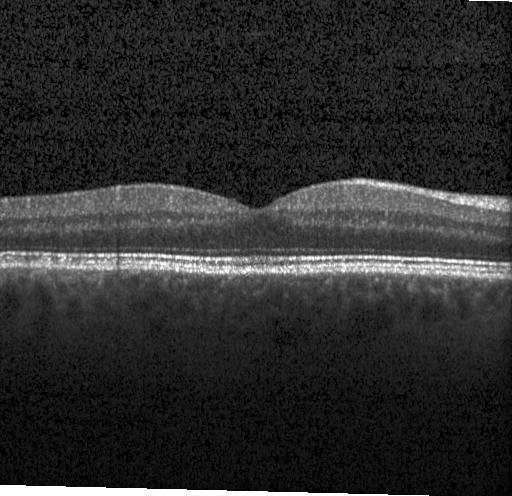
Horizontal scan through the fovea, retinal OCT B-scan.
Dx: no CNV, no DME, and no drusen.